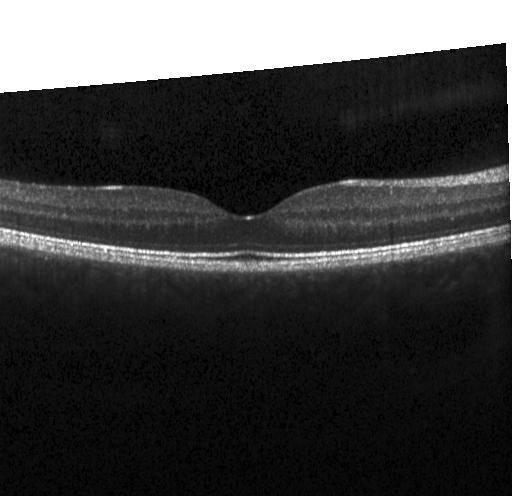
Spectral-domain OCT. Optical coherence tomography B-scan. Macular scan — Assessment: no CNV, DME, or drusen.